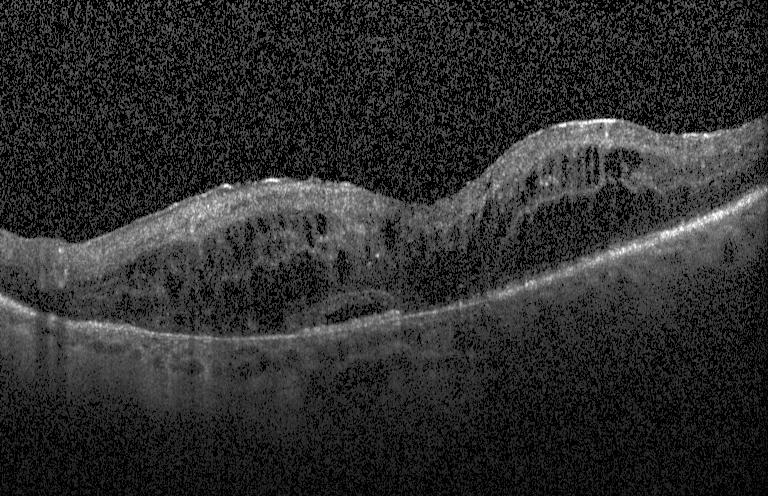
Instrument: Heidelberg Spectralis · retinal OCT B-scan · spectral-domain optical coherence tomography — Impression: choroidal neovascularization.